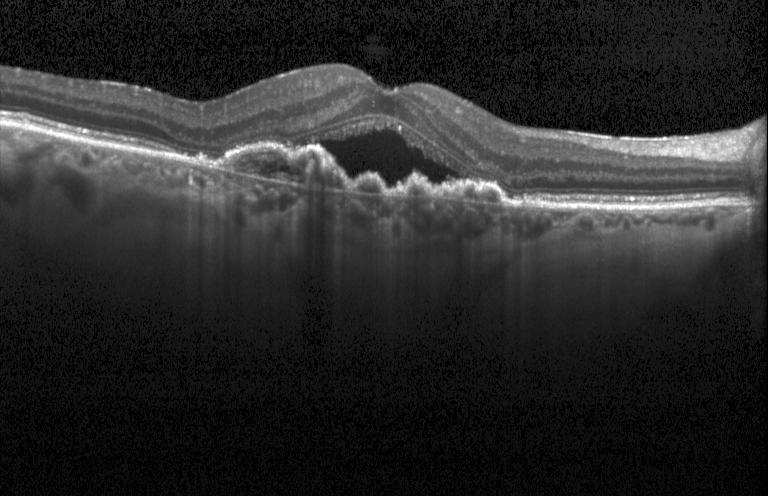

OCT scan showing choroidal neovascularization.